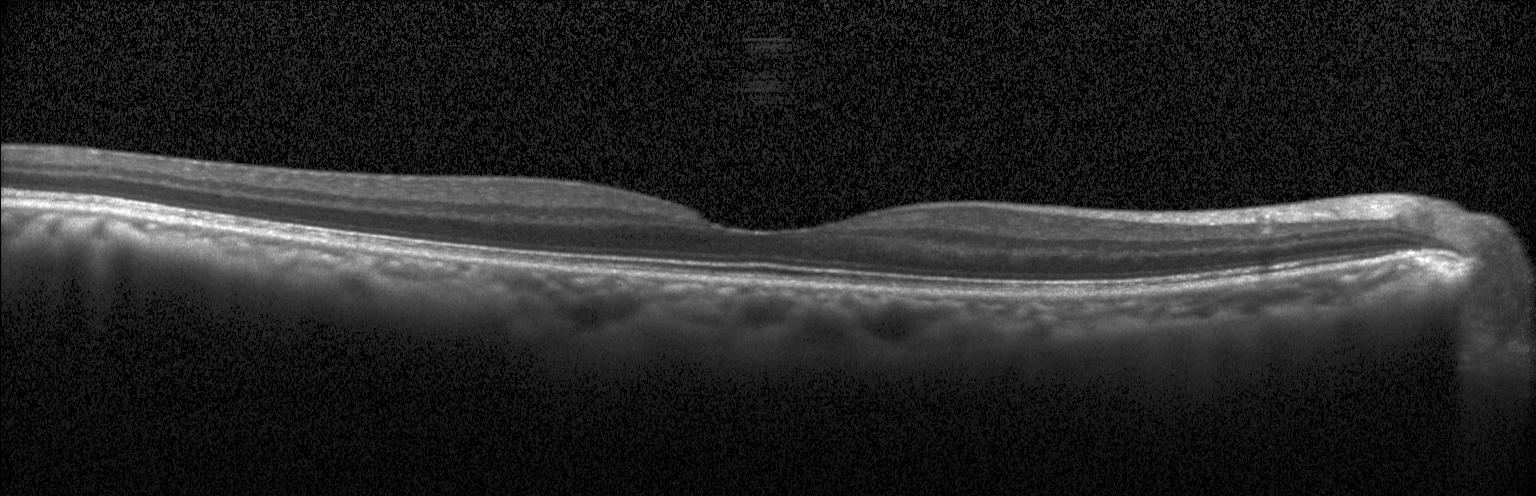 Spectral-domain OCT. Through the macula. Retinal OCT B-scan — Diagnosis: no choroidal neovascularization, no diabetic macular edema, and no drusen.